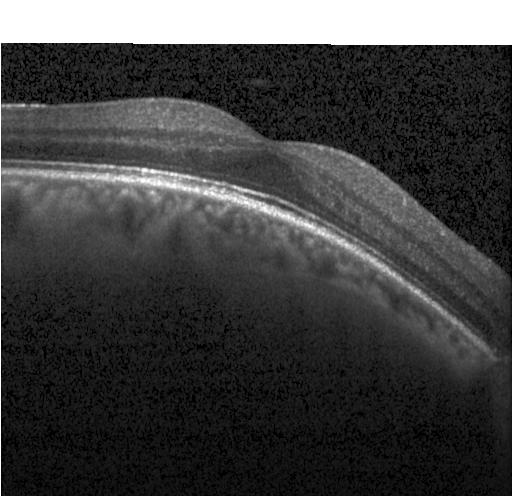
Dx: no choroidal neovascularization, no diabetic macular edema, and no drusen.